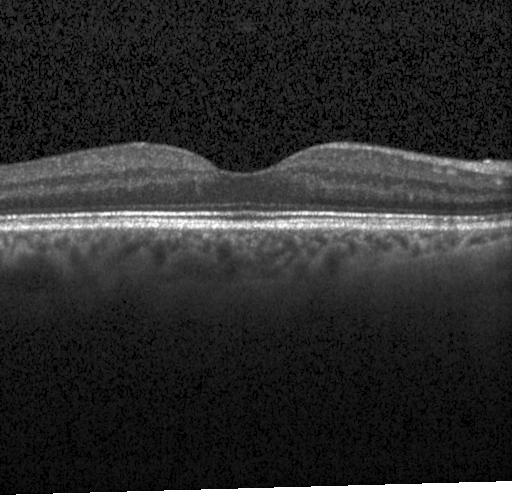

OCT line scan. Through the macula. Heidelberg Spectralis.
This B-scan demonstrates no choroidal neovascularization, diabetic macular edema, or drusen.